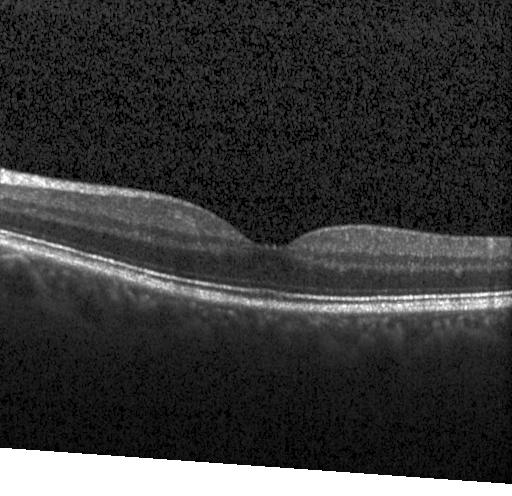
Dx: no choroidal neovascularization, no diabetic macular edema, and no drusen.